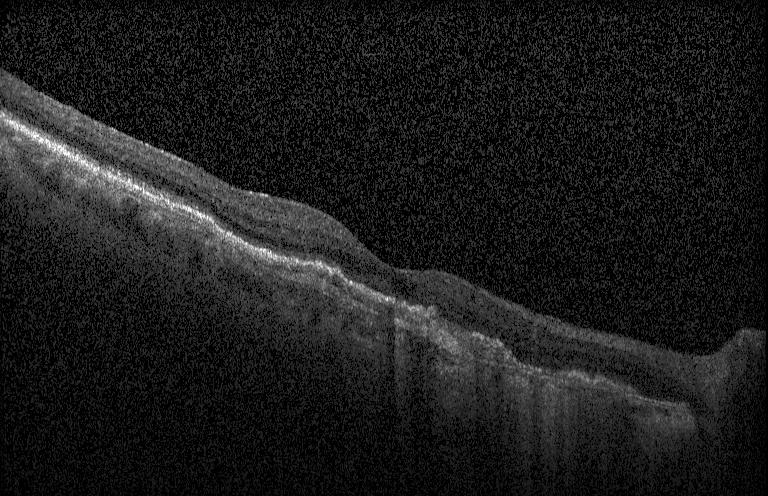

Retinal OCT B-scan · macular scan. Assessment: choroidal neovascularization (CNV).